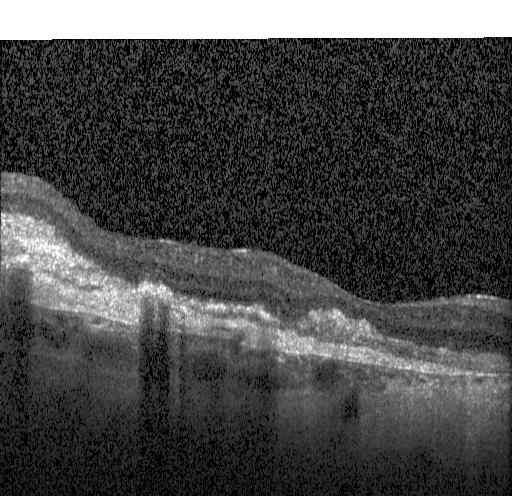 OCT finding: choroidal neovascularization.